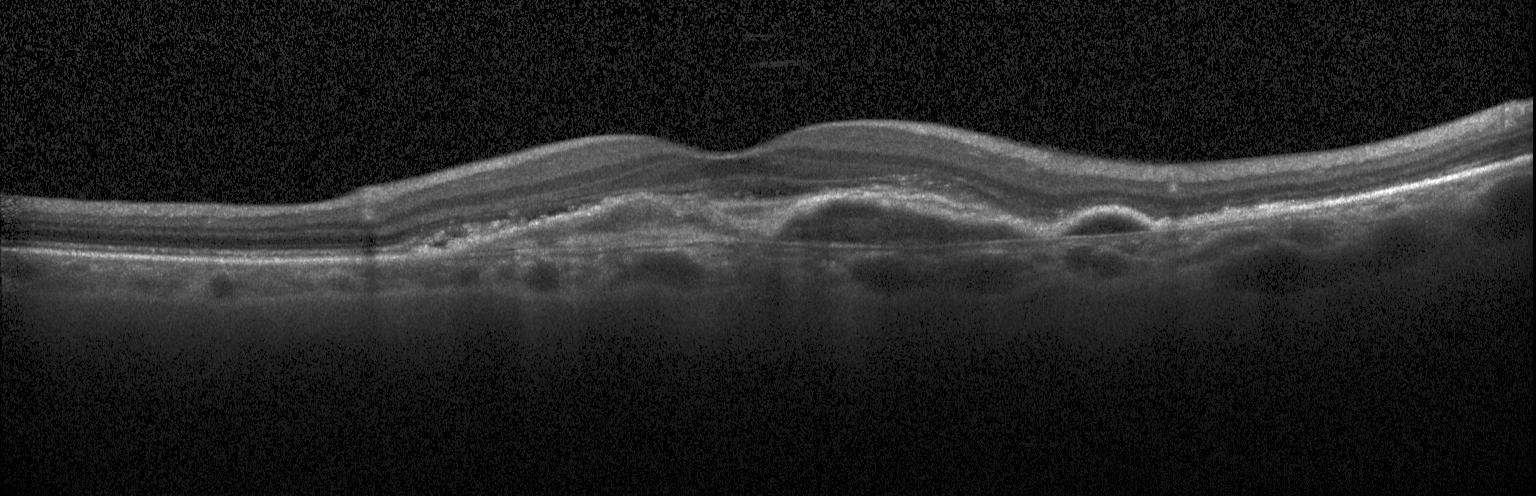
This B-scan demonstrates a choroidal neovascular membrane.